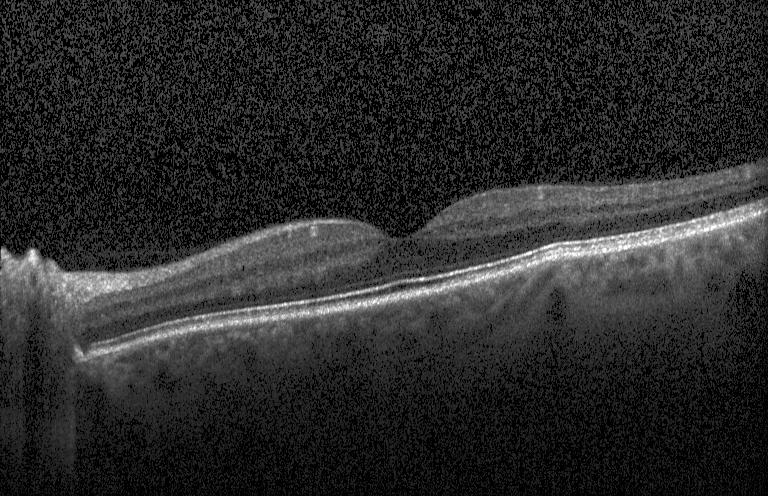 SD-OCT, centered on the fovea, Heidelberg Spectralis OCT system, retinal OCT B-scan
Impression: no choroidal neovascularization, diabetic macular edema, or drusen.